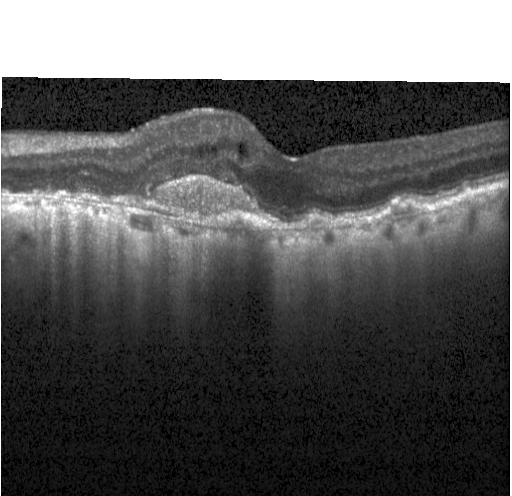

SD-OCT · macular scan · OCT line scan. Finding: a choroidal neovascular membrane.